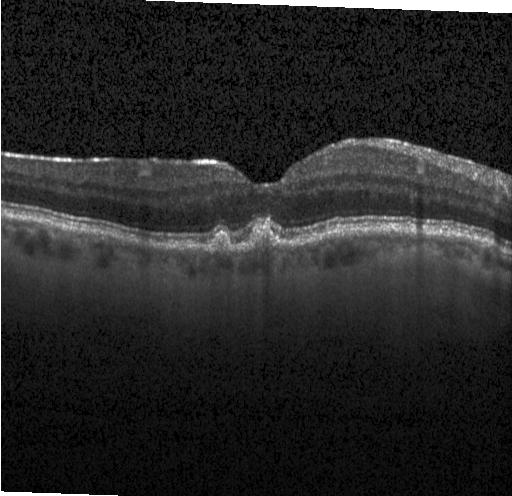
Heidelberg Spectralis; optical coherence tomography scan — Dx: drusen.